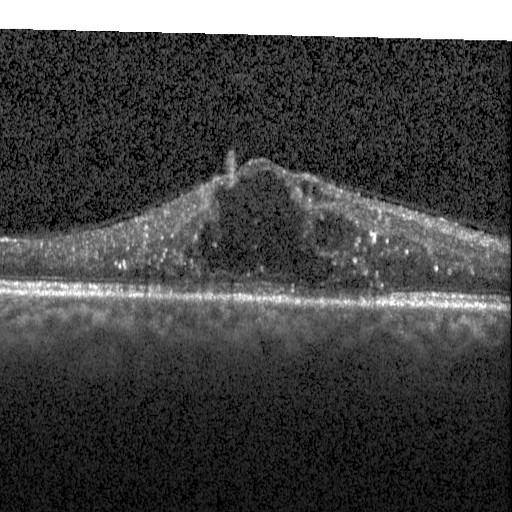 Optical coherence tomography B-scan — Dx: diabetic macular edema (DME).